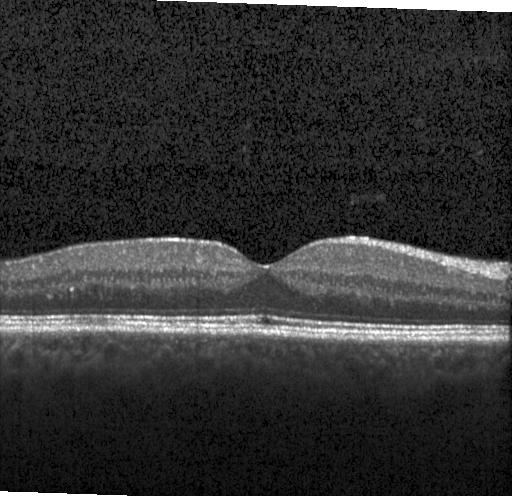 Centered on the fovea, retinal OCT cross-section. Finding: no choroidal neovascularization, no diabetic macular edema, and no drusen.